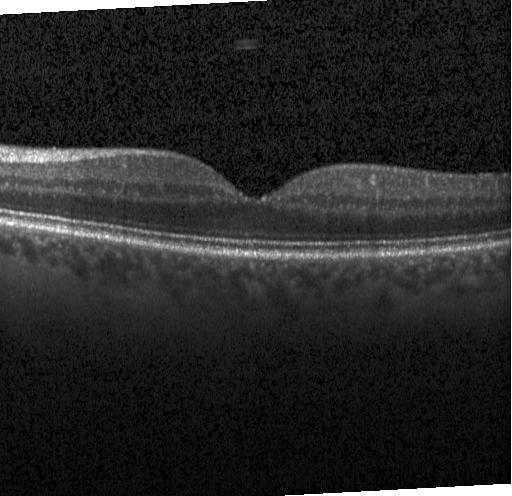

OCT B-scan — Macular OCT: no CNV, no DME, and no drusen.